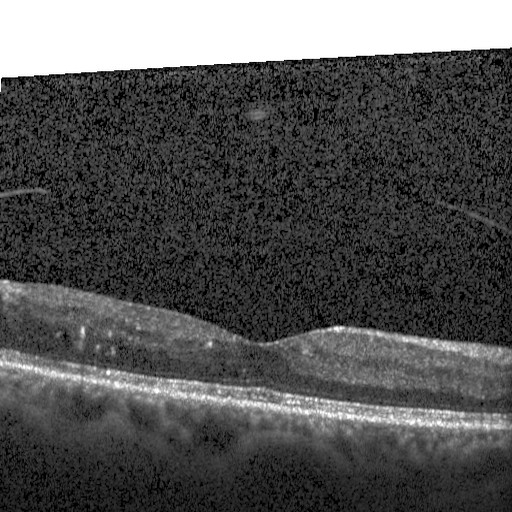 Instrument: Heidelberg Spectralis; retinal OCT cross-section; spectral-domain optical coherence tomography; through the macula. Impression: diabetic macular edema.